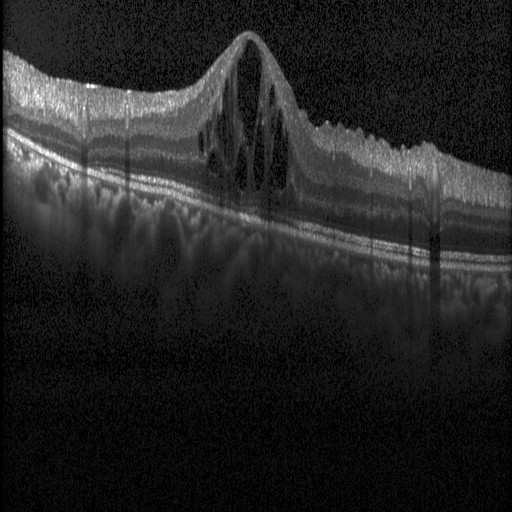 Macular OCT demonstrating diabetic macular edema (DME).